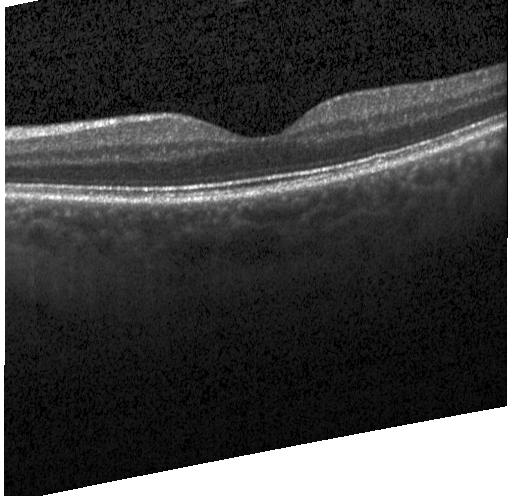
OCT finding: no choroidal neovascularization, diabetic macular edema, or drusen.